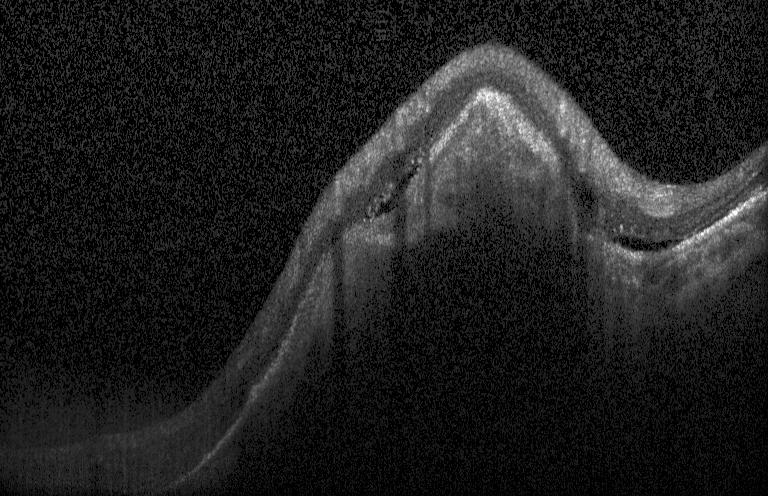
Impression: a choroidal neovascular membrane.